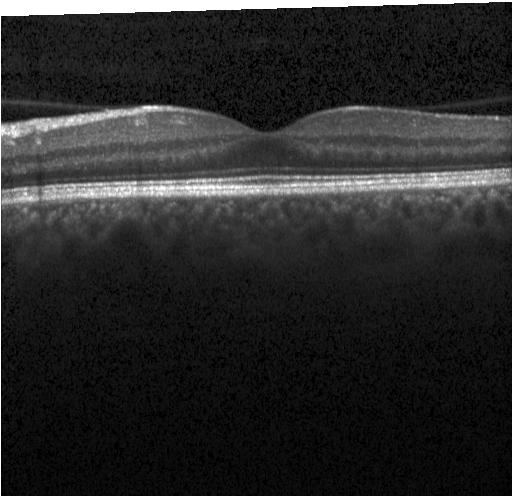
Heidelberg Spectralis. Fovea-centered. Spectral-domain optical coherence tomography. OCT B-scan
The scan shows no CNV, no DME, and no drusen.